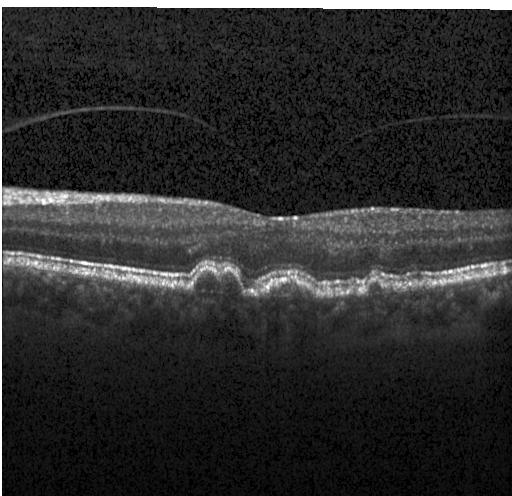
Optical coherence tomography scan; spectral-domain OCT. Diagnosis: sub-RPE drusenoid deposits.